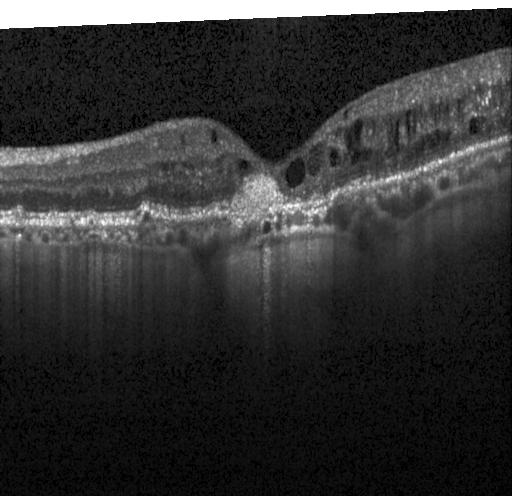
Dx: CNV.